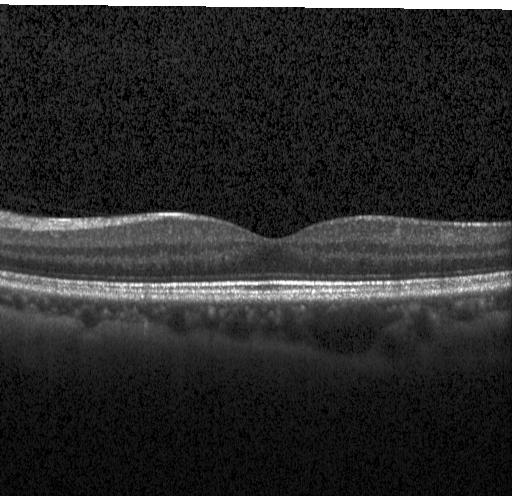

Finding: no evidence of choroidal neovascularization, diabetic macular edema, or drusen.